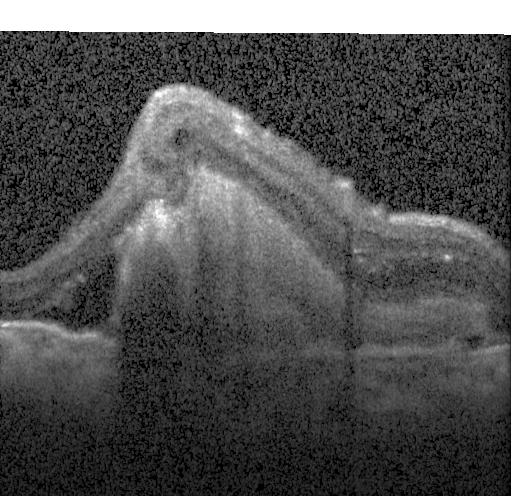
OCT finding: choroidal neovascularization.